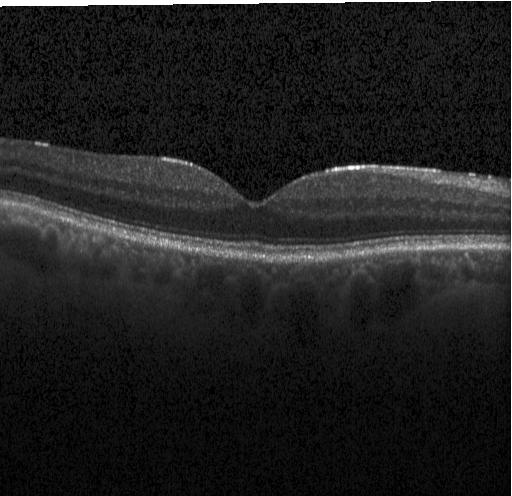 Centered on the fovea, OCT line scan, spectral-domain optical coherence tomography
Assessment: no choroidal neovascularization, no diabetic macular edema, and no drusen.